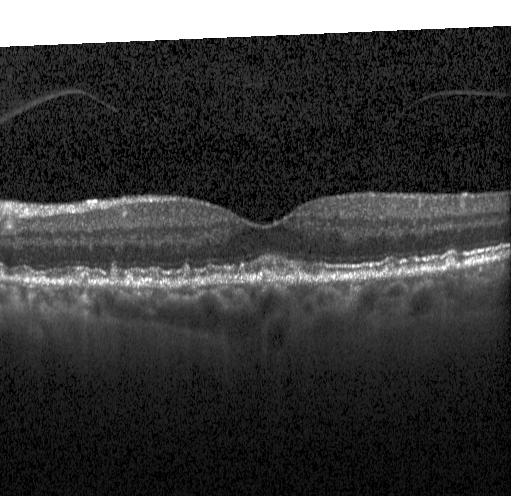
Retinal OCT B-scan. Instrument: Heidelberg Spectralis — The scan shows drusen.